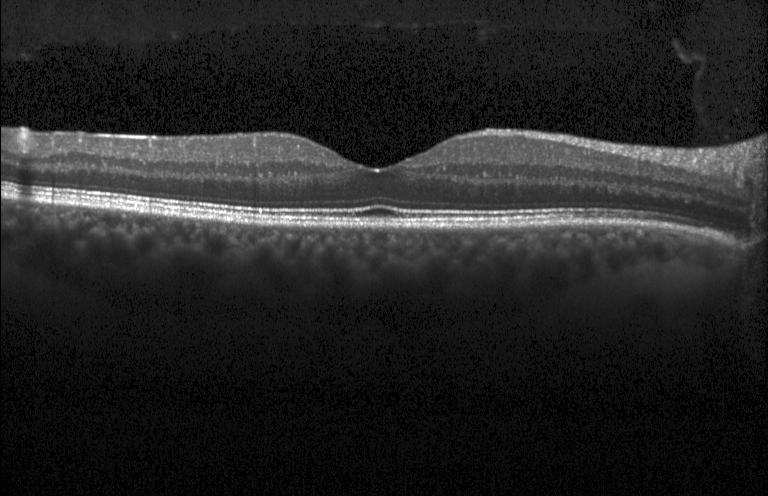
Assessment: no evidence of CNV, DME, or drusen.